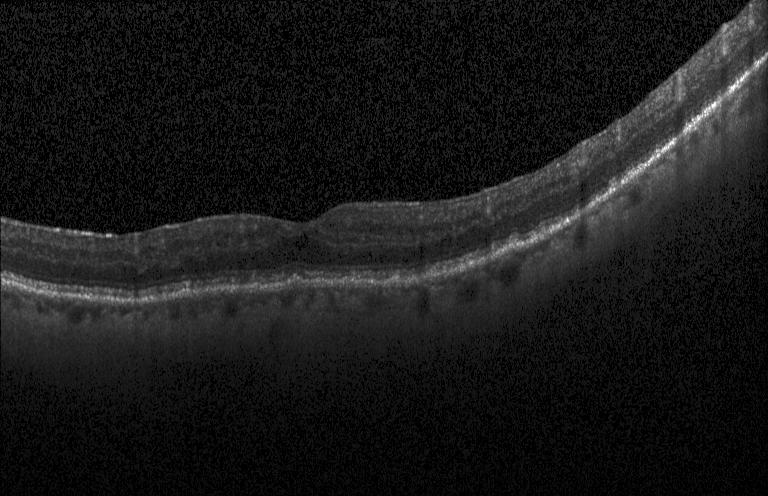 Retinal OCT B-scan · SD-OCT
Diagnosis: multiple drusen.